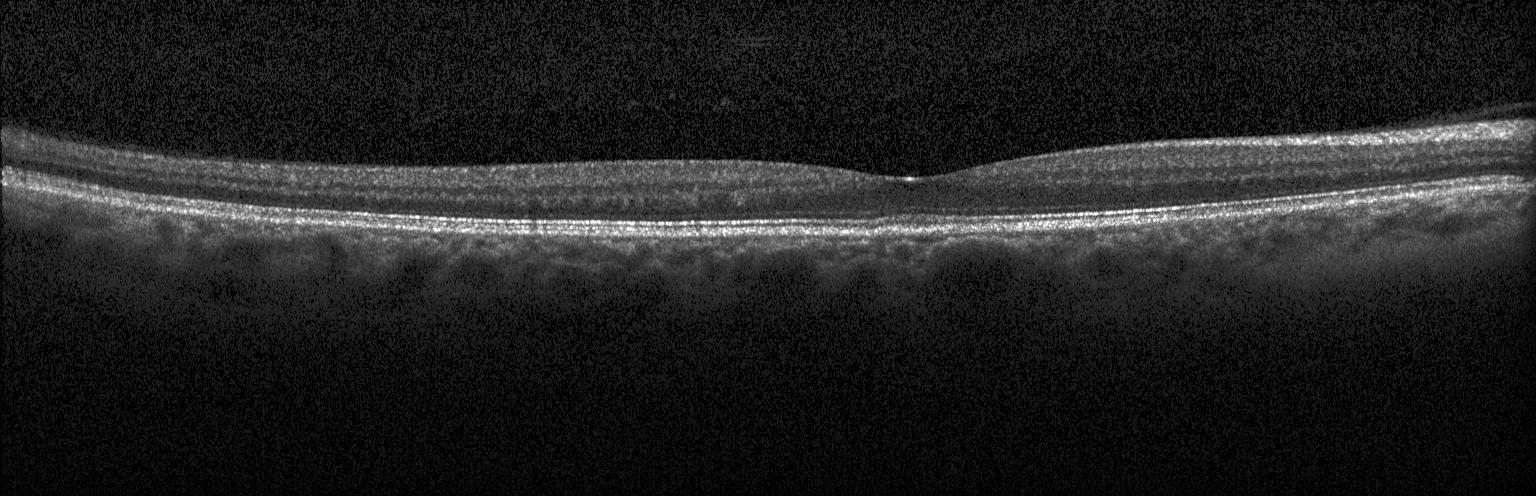

Spectral-domain optical coherence tomography. Horizontal scan through the fovea. Heidelberg Spectralis OCT system. Optical coherence tomography B-scan. This B-scan demonstrates no evidence of choroidal neovascularization, diabetic macular edema, or drusen.